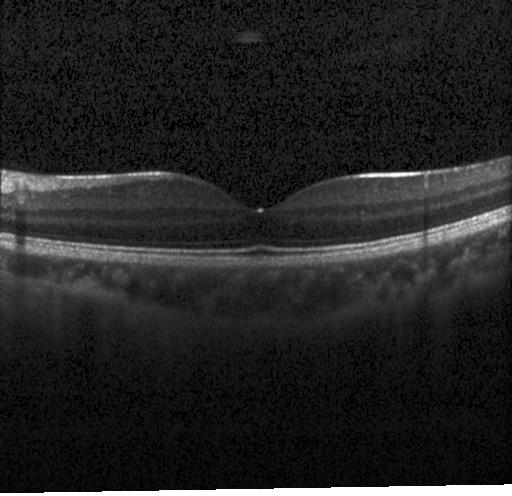 Dx: no evidence of choroidal neovascularization, diabetic macular edema, or drusen.